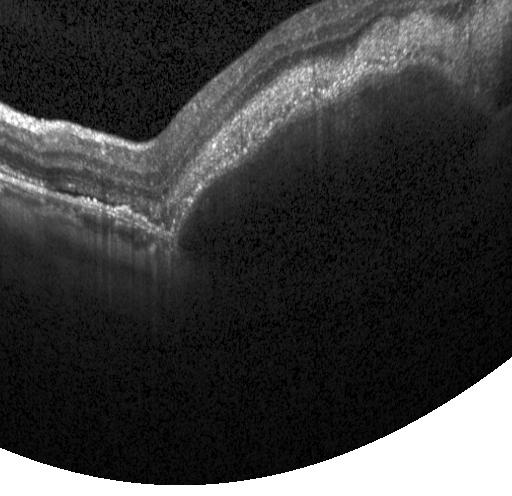

The scan shows a choroidal neovascular membrane.